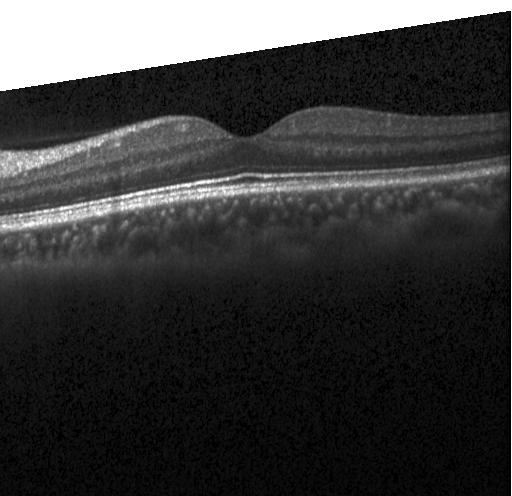 Impression: no choroidal neovascularization, diabetic macular edema, or drusen.